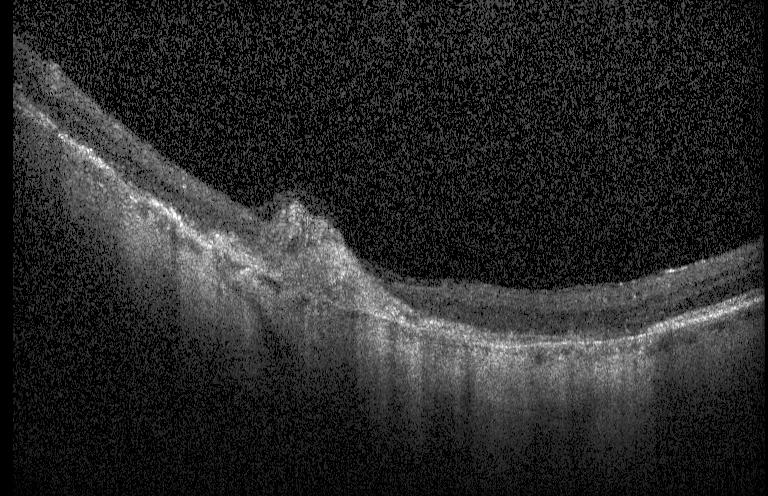
Assessment: a choroidal neovascular membrane.